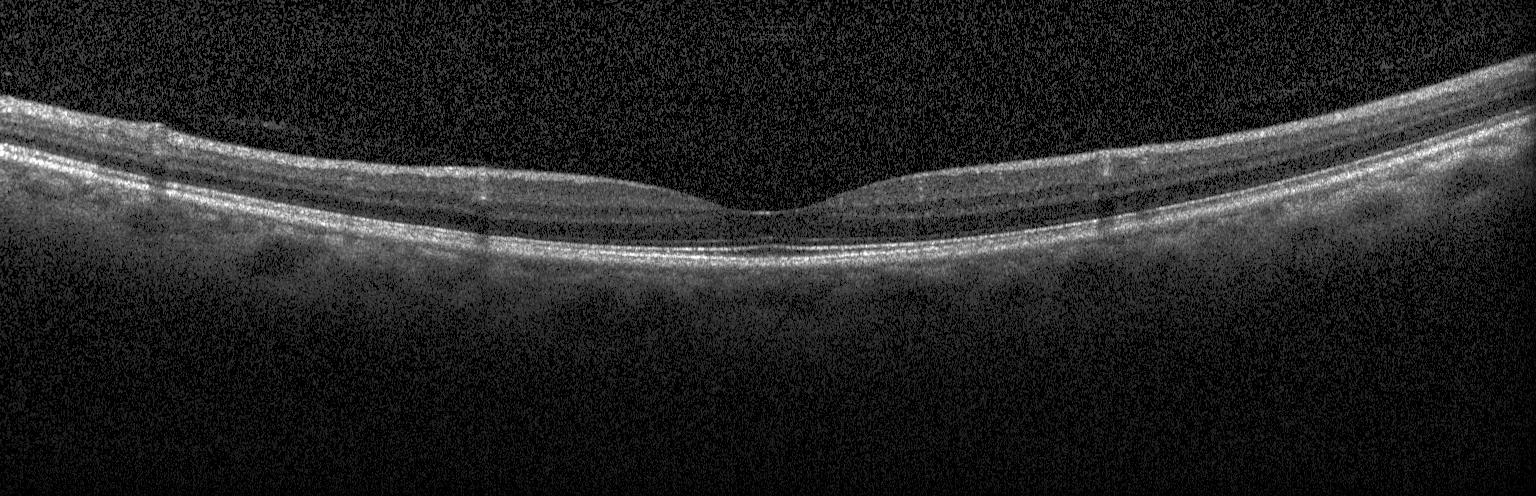 Macular OCT demonstrating no evidence of choroidal neovascularization, diabetic macular edema, or drusen.